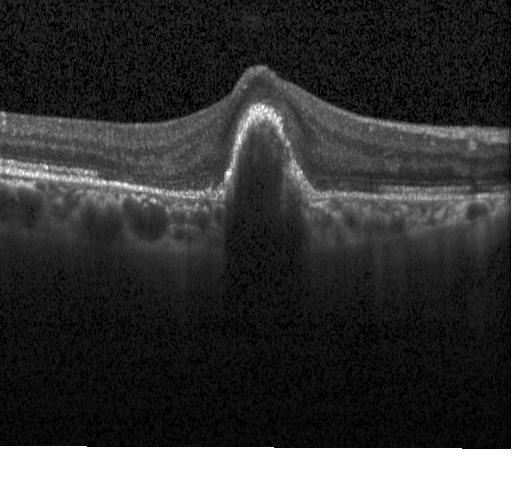
OCT line scan · Heidelberg Spectralis OCT system · horizontal scan through the fovea · spectral-domain optical coherence tomography
Dx: CNV.